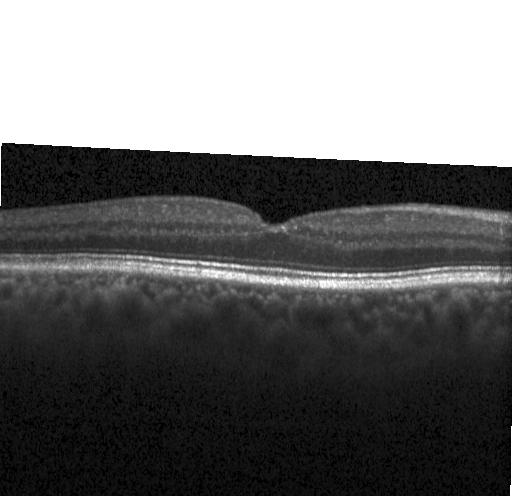
OCT finding: no choroidal neovascularization, no diabetic macular edema, and no drusen.